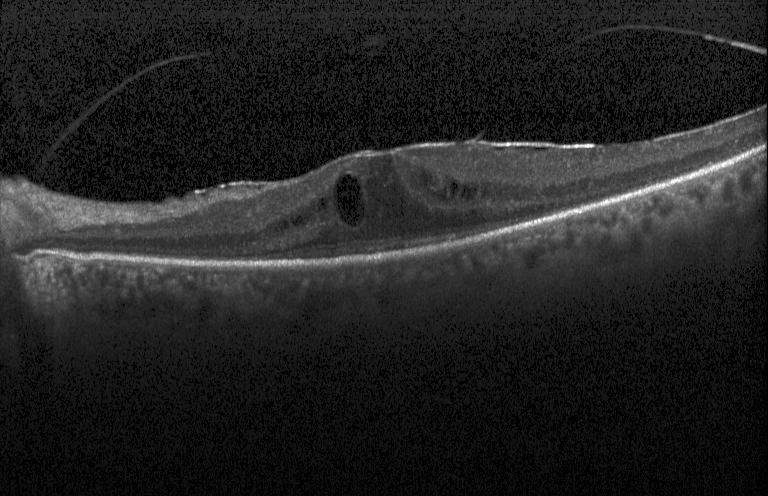
Spectral-domain optical coherence tomography; retinal OCT B-scan. Impression: DME.